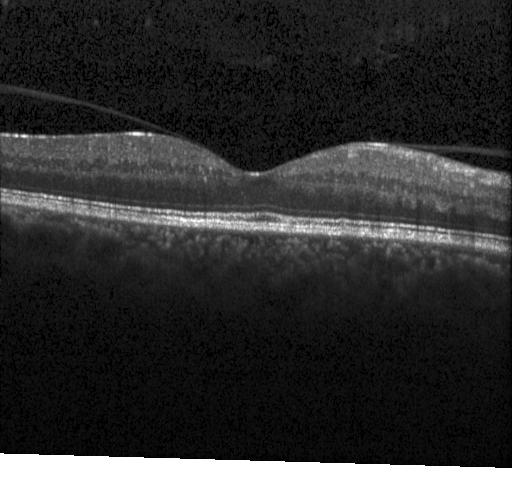
Optical coherence tomography B-scan
Impression: no CNV, no DME, and no drusen.